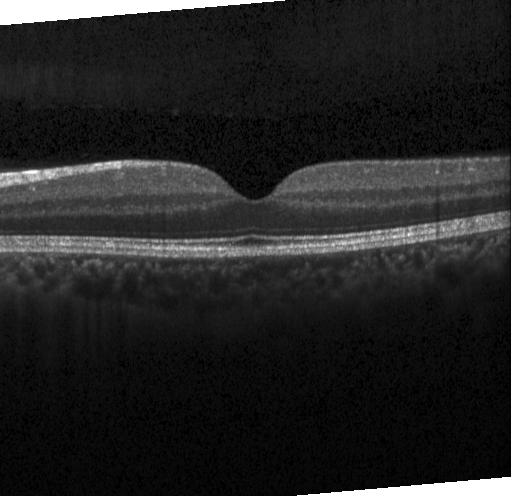

Spectral-domain optical coherence tomography, retinal OCT B-scan, fovea-centered — Finding: no evidence of choroidal neovascularization, diabetic macular edema, or drusen.